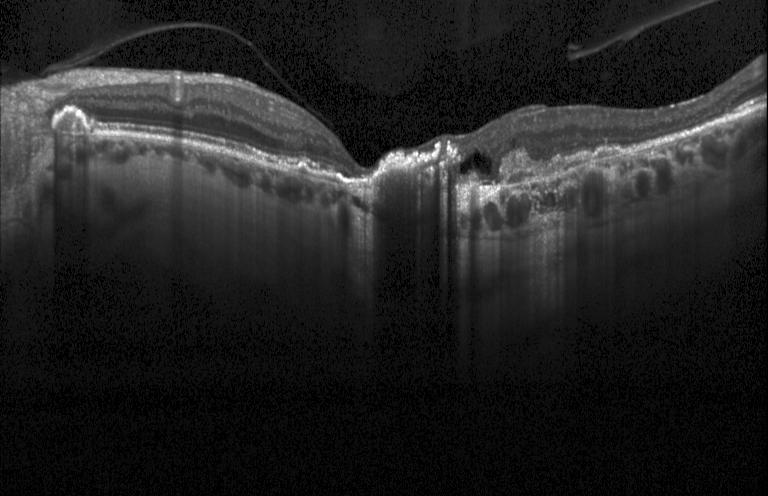
Retinal OCT B-scan
Impression: a choroidal neovascular membrane.